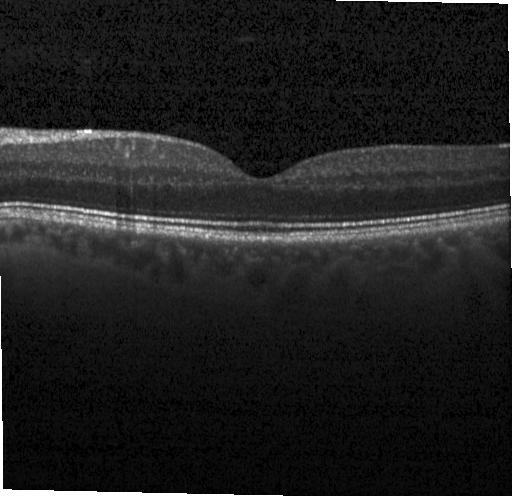
OCT B-scan; spectral-domain OCT. This B-scan demonstrates no choroidal neovascularization, diabetic macular edema, or drusen.